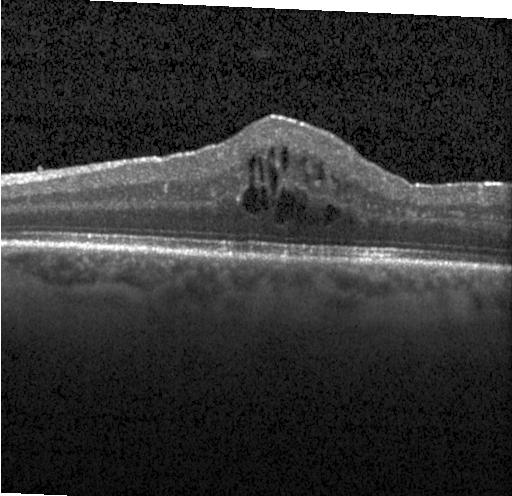
The scan shows diabetic macular edema.